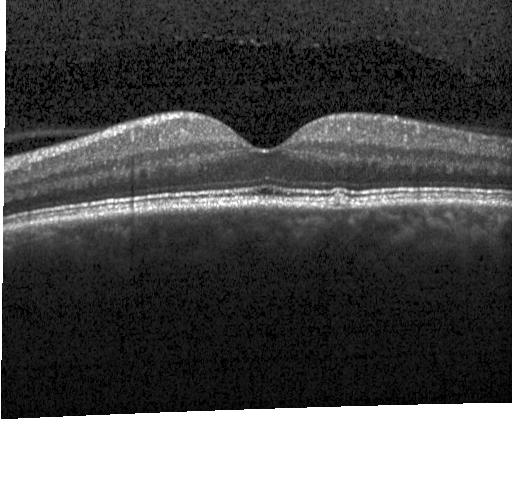 OCT line scan
OCT finding: sub-RPE drusenoid deposits.